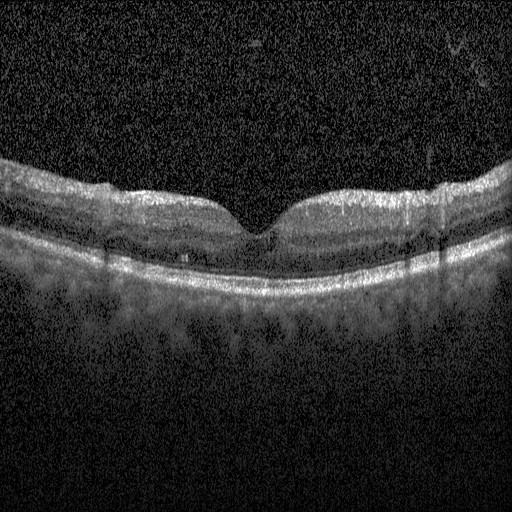 Spectral-domain OCT, optical coherence tomography scan — Diagnosis: diabetic macular edema (DME).